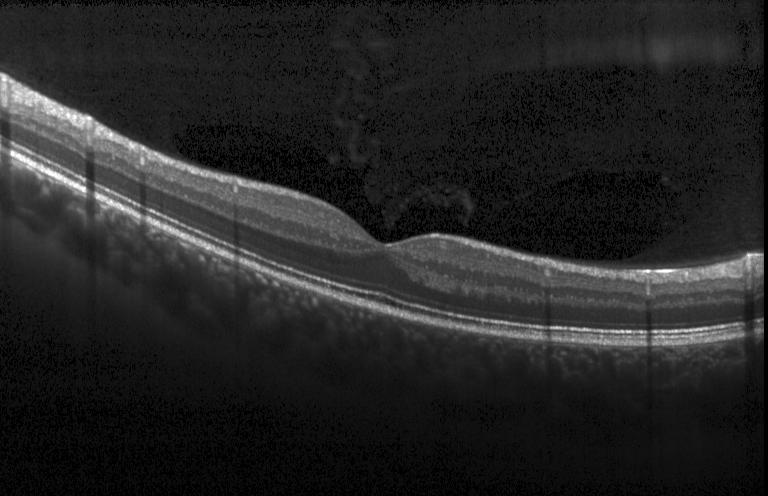 Optical coherence tomography scan. Centered on the fovea
Dx: no choroidal neovascularization, no diabetic macular edema, and no drusen.